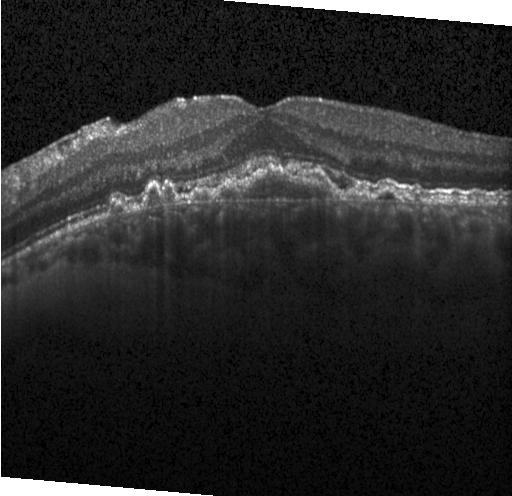 Finding: choroidal neovascularization (CNV).